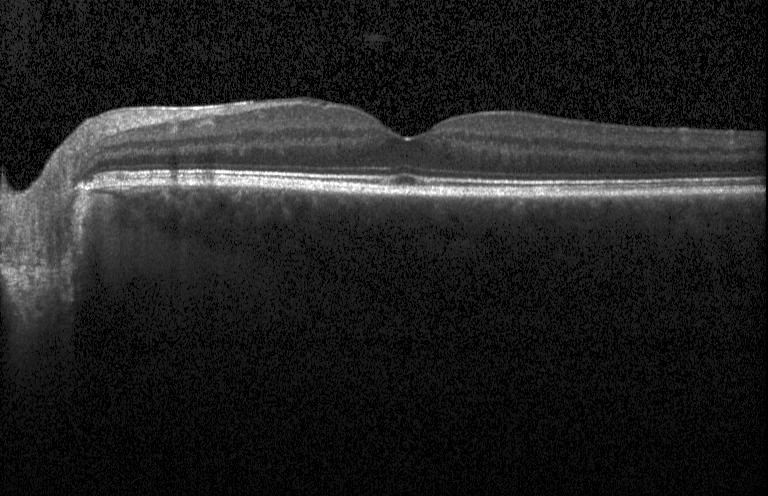 Retinal OCT cross-section showing neither CNV, DME, nor drusen.